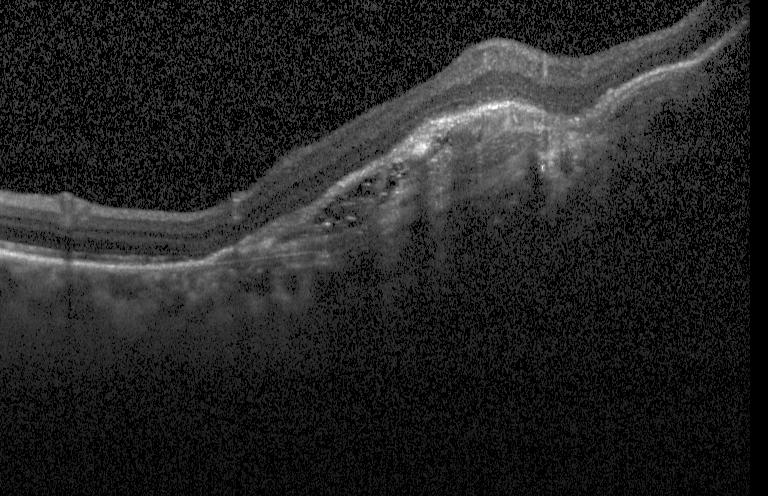 OCT B-scan showing choroidal neovascularization.